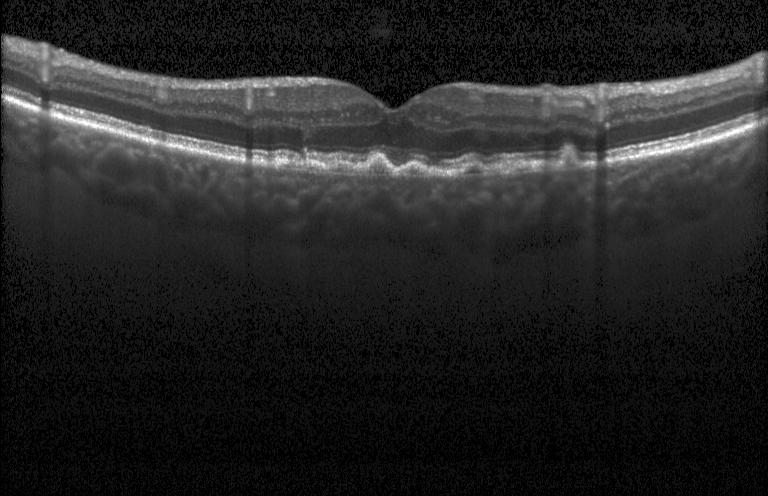 Retinal OCT cross-section; through the macula; acquired on a Heidelberg Spectralis; spectral-domain optical coherence tomography. Impression: drusen.